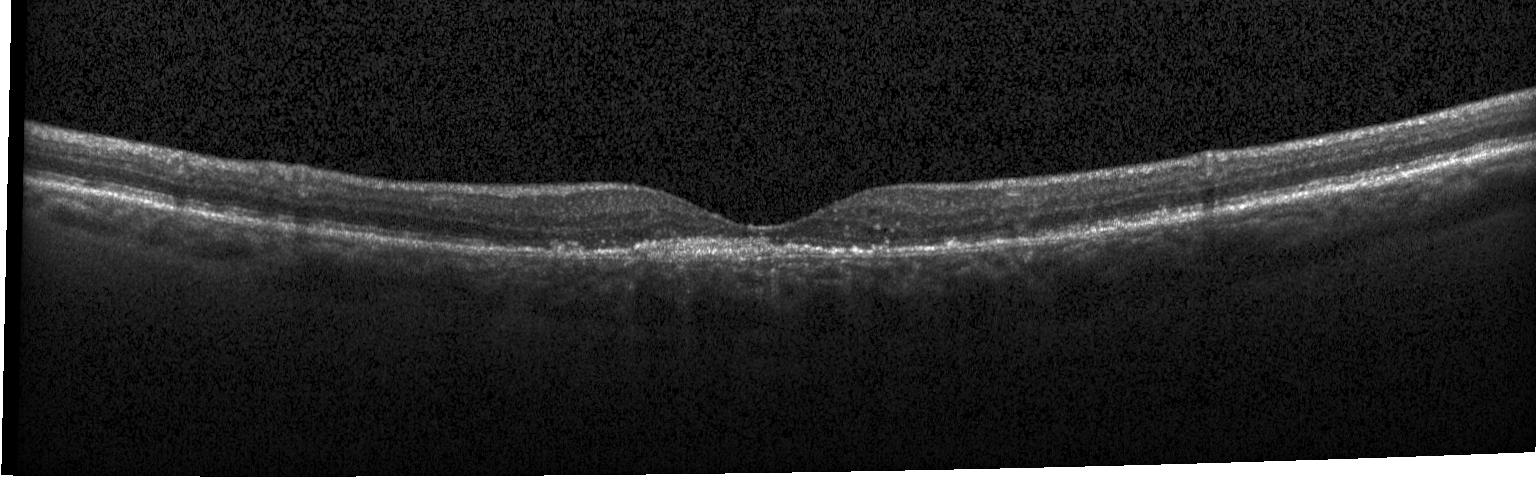
Heidelberg Spectralis OCT system · retinal OCT cross-section · fovea-centered
OCT finding: a choroidal neovascular membrane.